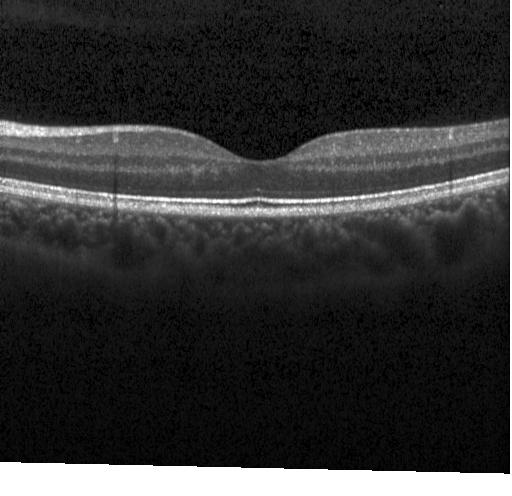
OCT B-scan · spectral-domain optical coherence tomography · horizontal scan through the fovea.
Impression: no choroidal neovascularization, no diabetic macular edema, and no drusen.